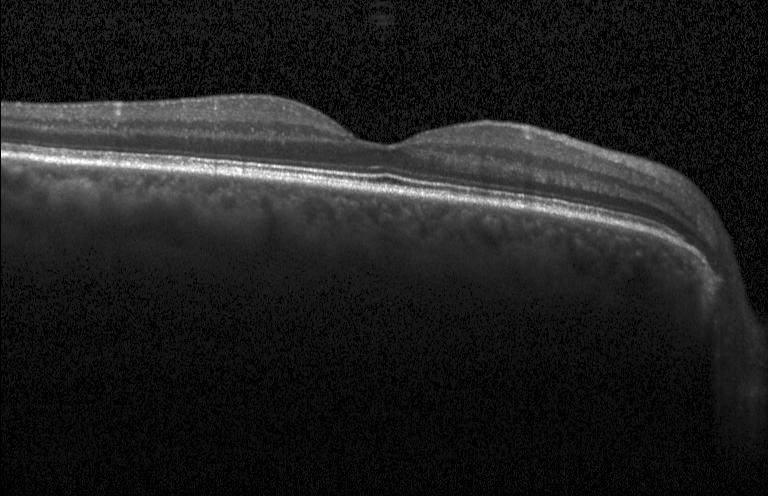
Optical coherence tomography B-scan · instrument: Heidelberg Spectralis
No CNV, no DME, and no drusen.